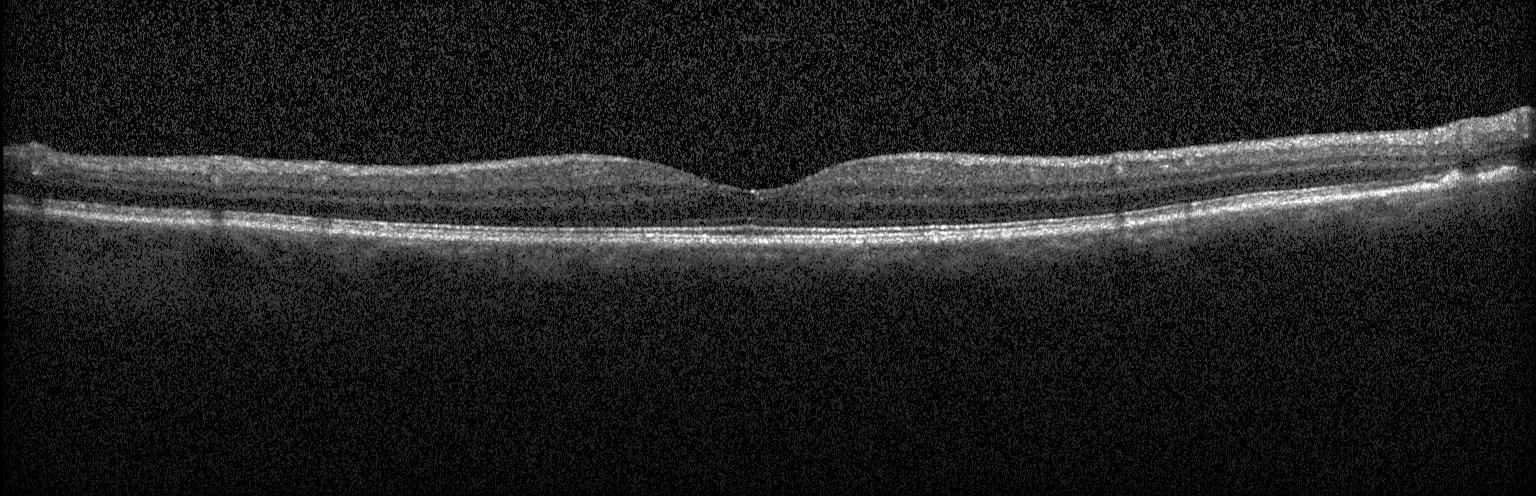 SD-OCT, OCT B-scan, instrument: Heidelberg Spectralis, horizontal scan through the fovea. Impression: no evidence of CNV, DME, or drusen.